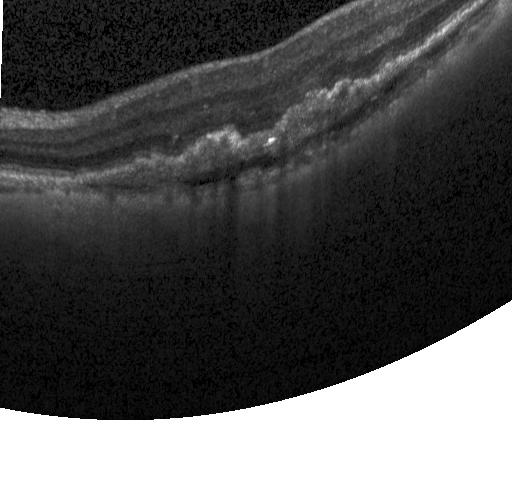
Macular OCT demonstrating choroidal neovascularization (CNV).